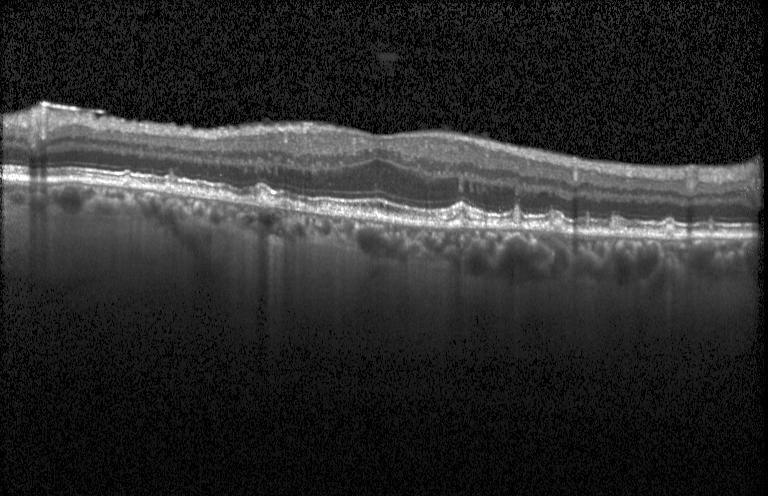

Retinal OCT cross-section showing drusen.